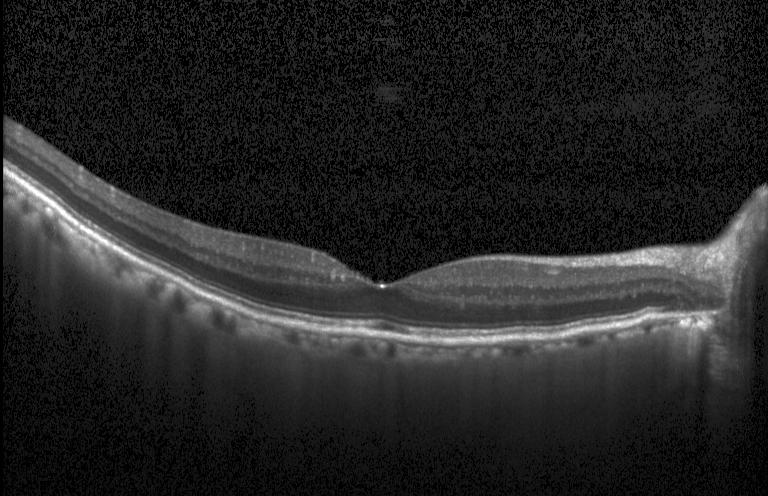

Horizontal scan through the fovea. SD-OCT. OCT B-scan. Instrument: Heidelberg Spectralis. OCT finding: no evidence of CNV, DME, or drusen.